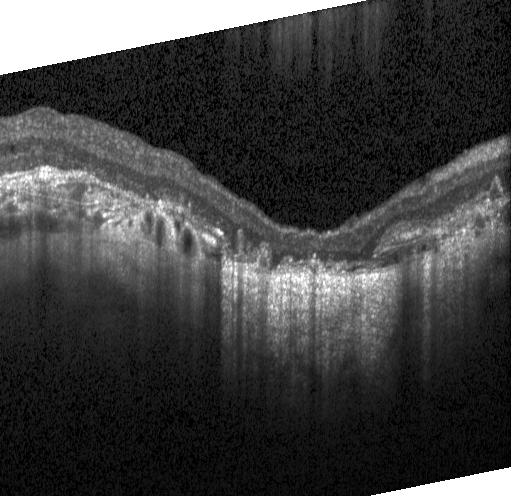

OCT line scan. Macular OCT: a choroidal neovascular membrane.